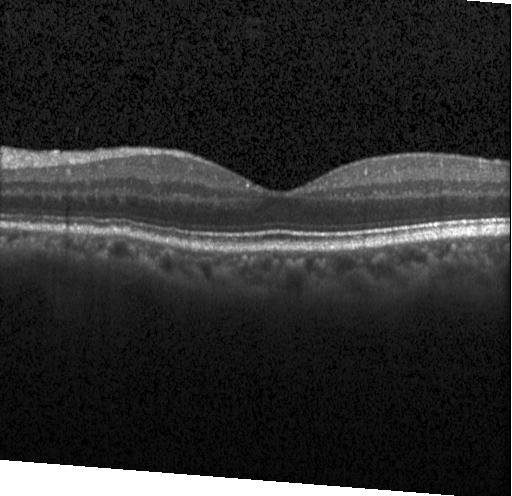
Macular OCT demonstrating no CNV, DME, or drusen.